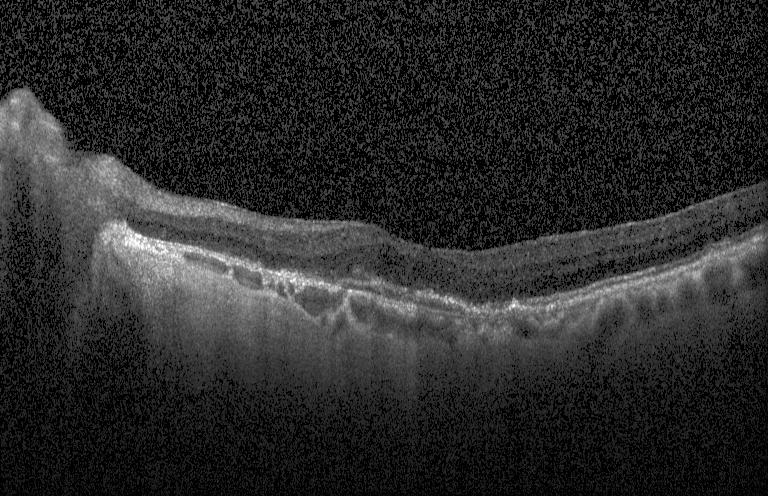

OCT B-scan showing choroidal neovascularization.